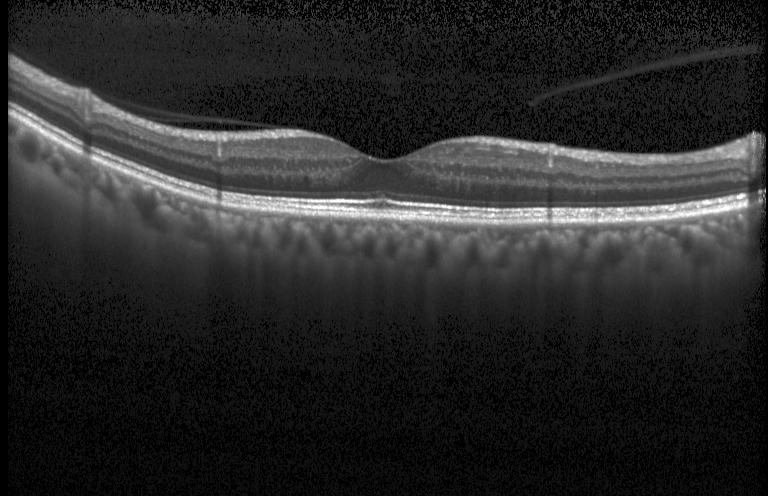
Diagnosis: no choroidal neovascularization, diabetic macular edema, or drusen.